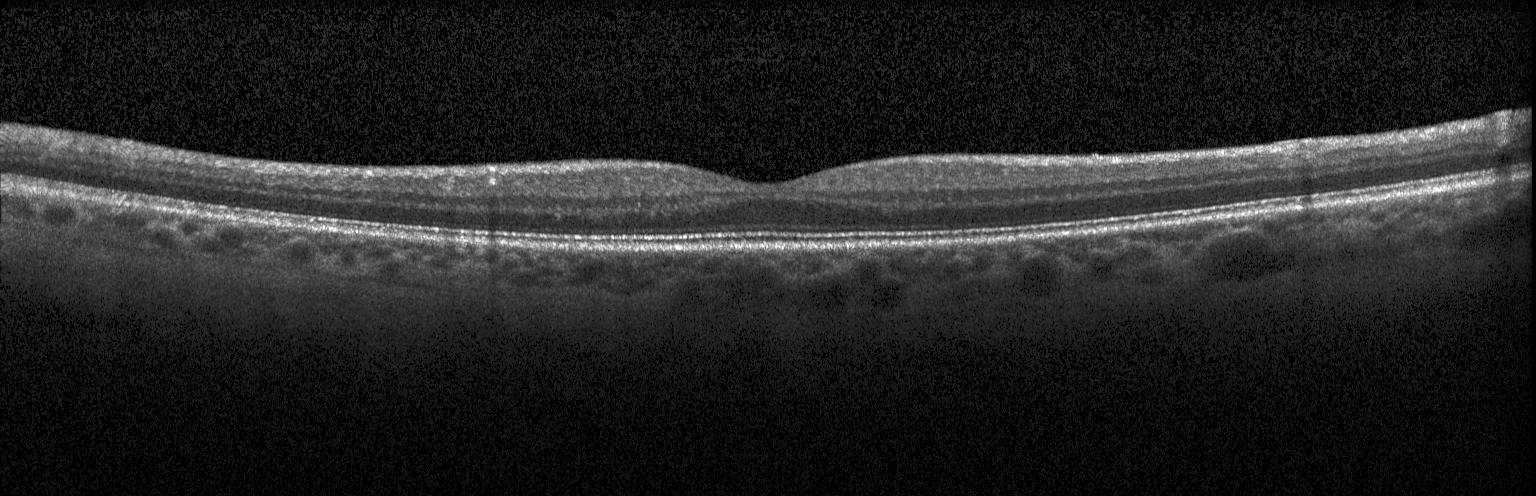 Assessment: no choroidal neovascularization, no diabetic macular edema, and no drusen.